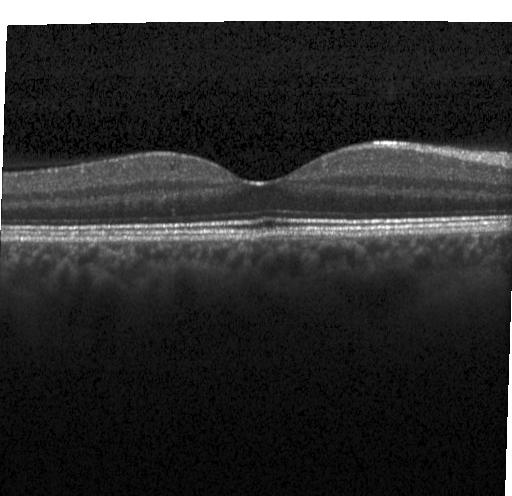 OCT finding: no CNV, DME, or drusen.